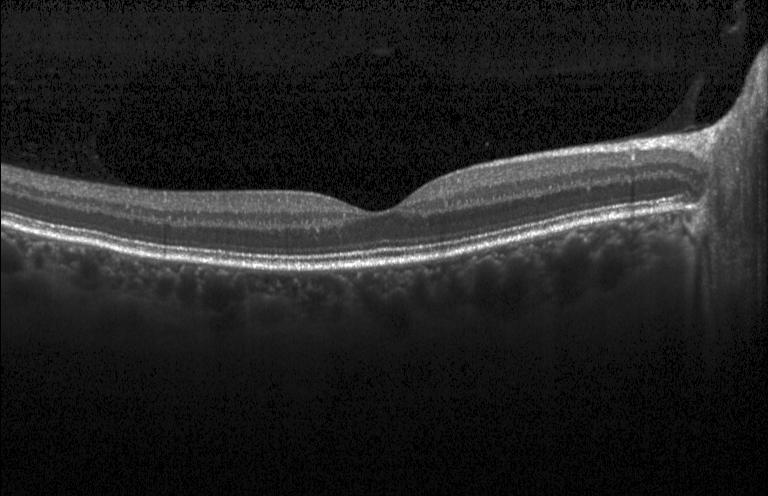

Spectral-domain optical coherence tomography, retinal OCT B-scan, Heidelberg Spectralis OCT system, centered on the fovea.
Diagnosis: no evidence of choroidal neovascularization, diabetic macular edema, or drusen.